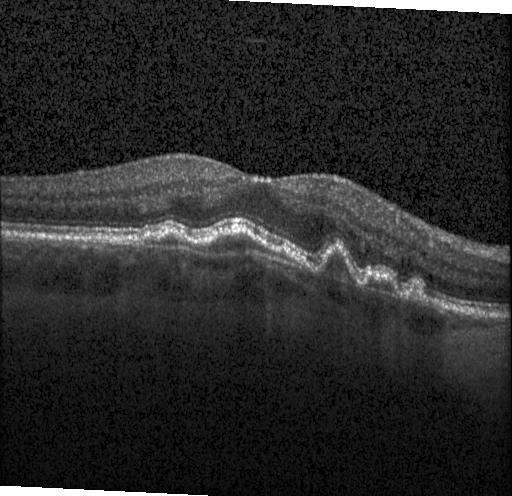 Centered on the fovea; Heidelberg Spectralis OCT system; spectral-domain OCT; OCT B-scan
Dx: a choroidal neovascular membrane.